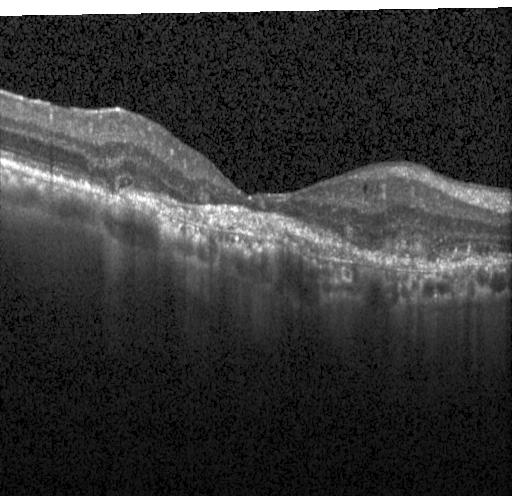
Optical coherence tomography scan · spectral-domain optical coherence tomography · centered on the fovea · acquired on a Heidelberg Spectralis.
The scan shows a choroidal neovascular membrane.